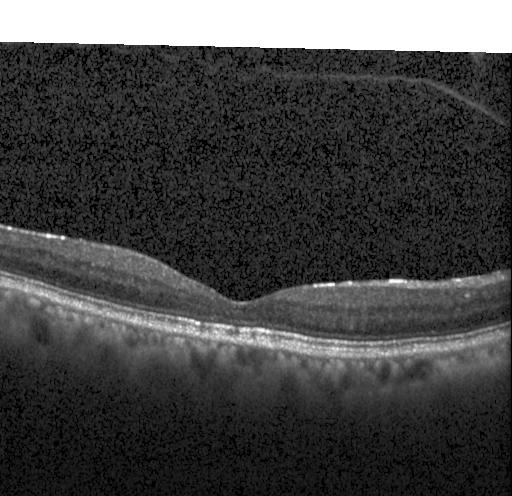

Fovea-centered · Heidelberg Spectralis · spectral-domain optical coherence tomography · OCT B-scan. No choroidal neovascularization, no diabetic macular edema, and no drusen.